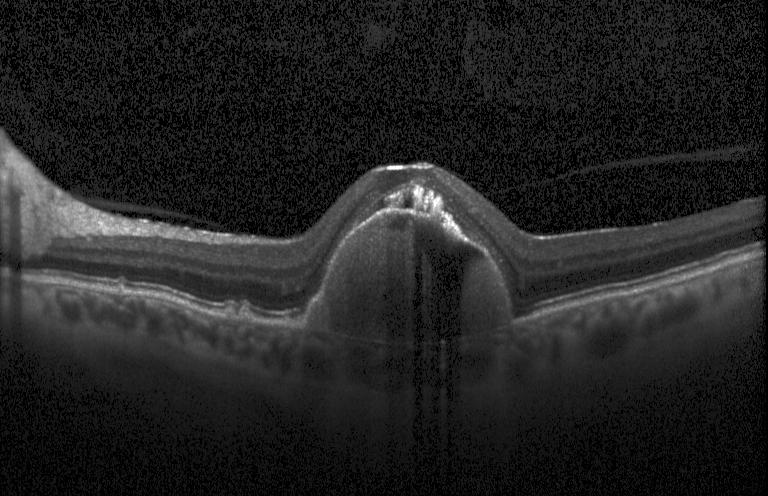 OCT B-scan.
Finding: choroidal neovascularization.